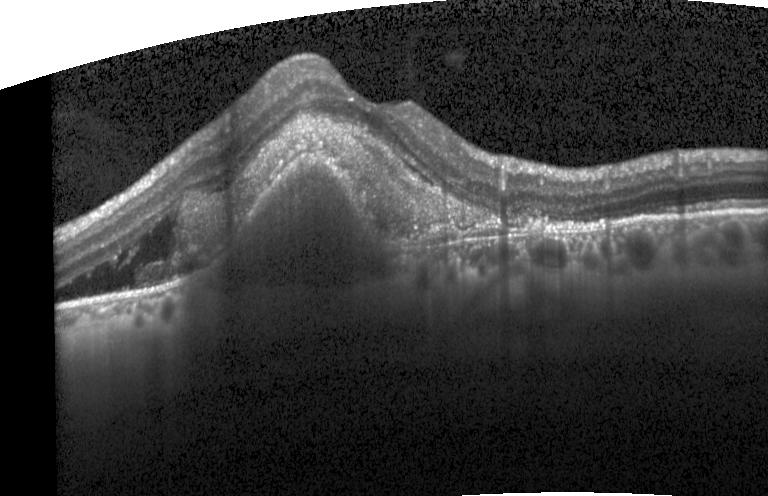

Acquired on a Heidelberg Spectralis; OCT line scan; spectral-domain optical coherence tomography; macular scan
Diagnosis: choroidal neovascularization.